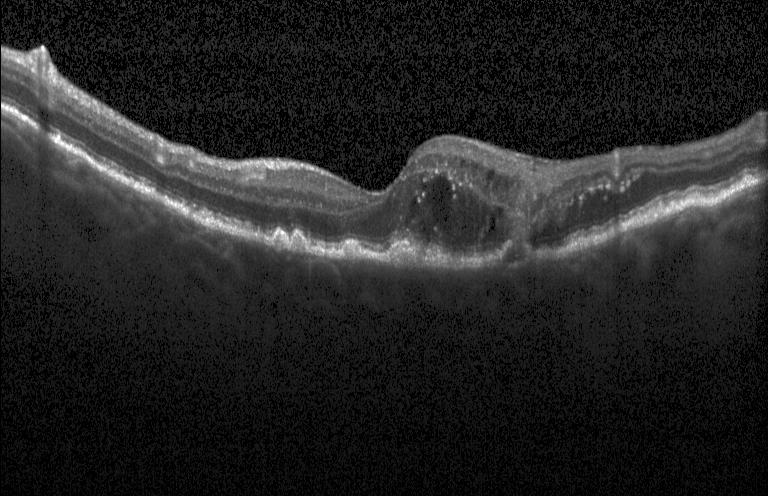 Optical coherence tomography scan; spectral-domain OCT.
Macular OCT: a choroidal neovascular membrane.